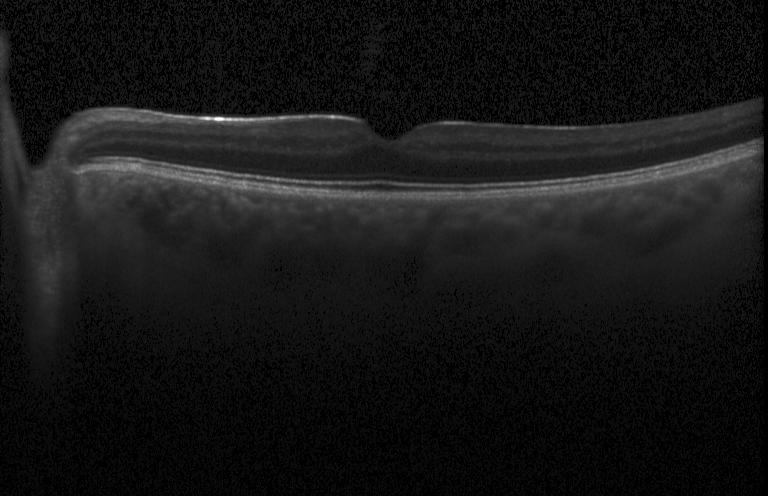 Impression: neither choroidal neovascularization, diabetic macular edema, nor drusen.